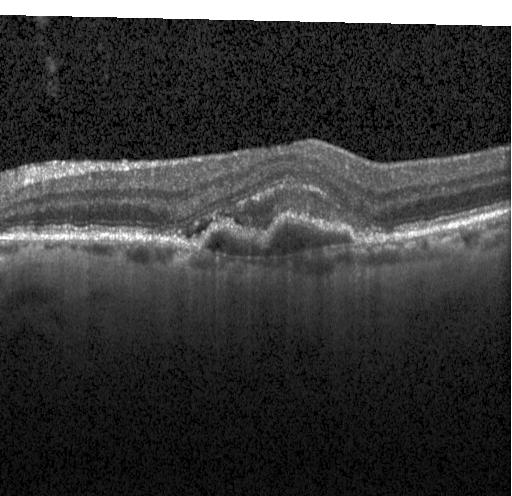

Retinal OCT B-scan, Heidelberg Spectralis OCT system.
OCT finding: a choroidal neovascular membrane.